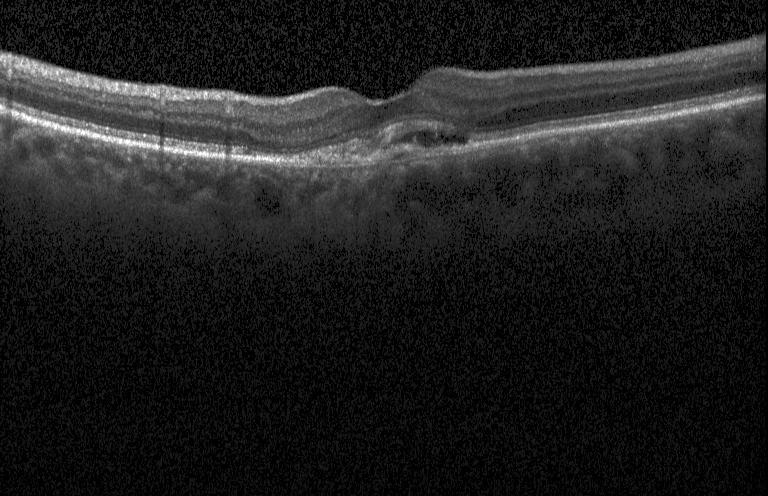
Optical coherence tomography scan.
This B-scan demonstrates CNV.